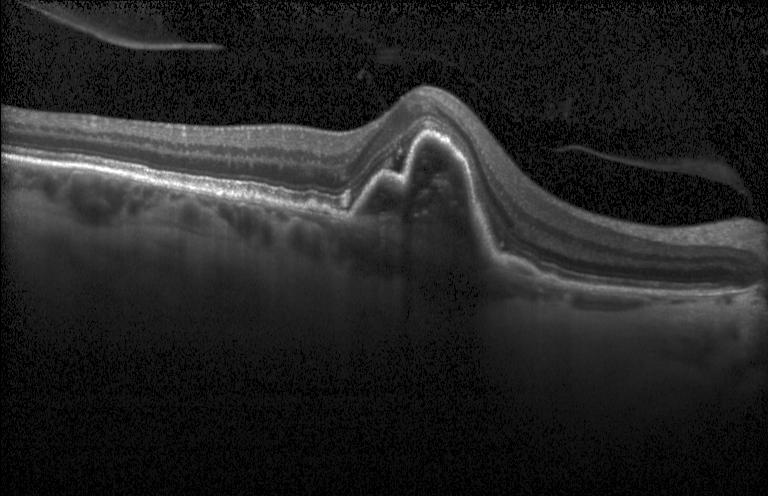 Optical coherence tomography B-scan, SD-OCT, instrument: Heidelberg Spectralis, fovea-centered
Finding: a choroidal neovascular membrane.